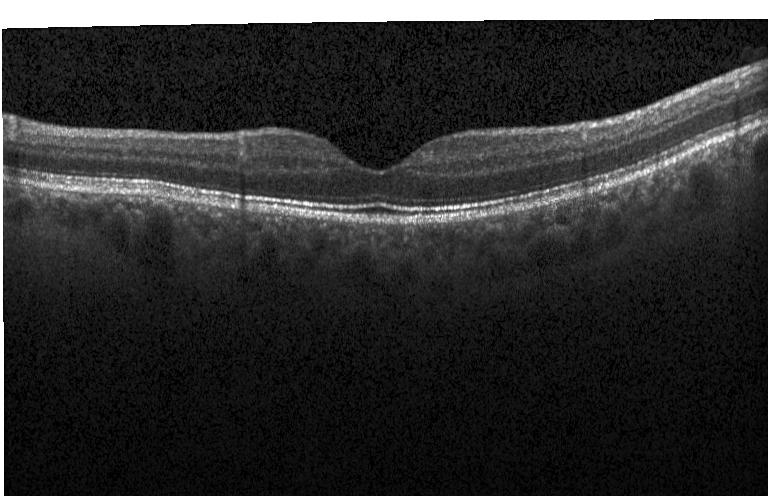
Dx: neither CNV, DME, nor drusen.